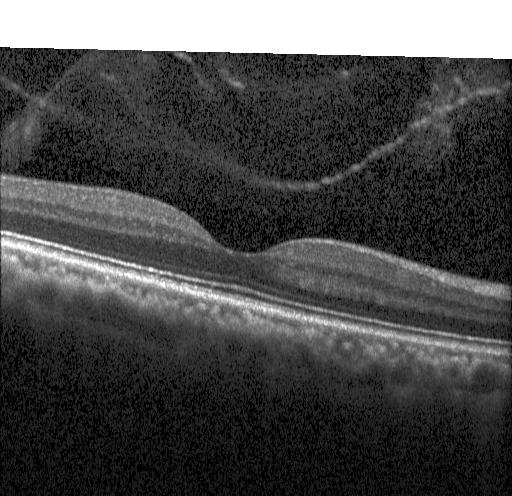

Spectral-domain OCT. Horizontal scan through the fovea. Retinal OCT cross-section.
Assessment: neither choroidal neovascularization, diabetic macular edema, nor drusen.